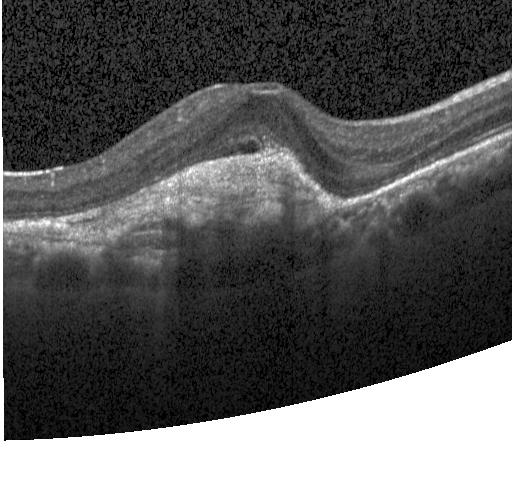
Spectral-domain OCT · optical coherence tomography scan · fovea-centered. Assessment: choroidal neovascularization (CNV).